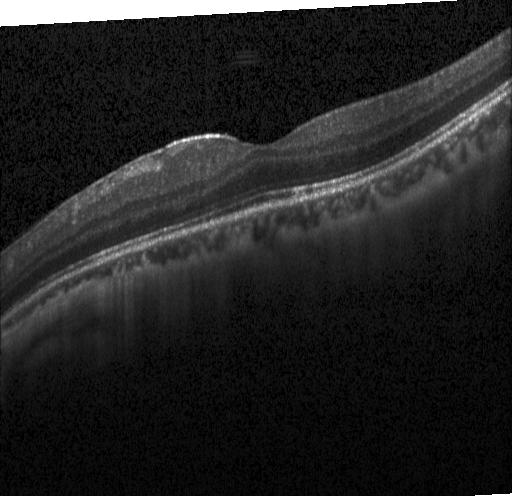

Acquired on a Heidelberg Spectralis. OCT B-scan.
OCT finding: no CNV, DME, or drusen.